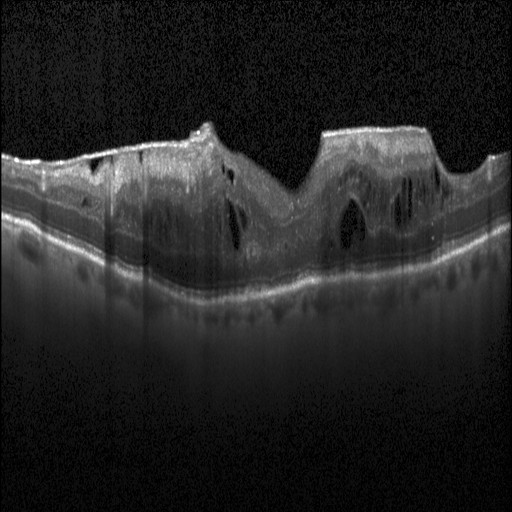 Retinal OCT cross-section · acquired on a Heidelberg Spectralis · spectral-domain OCT. Dx: DME.